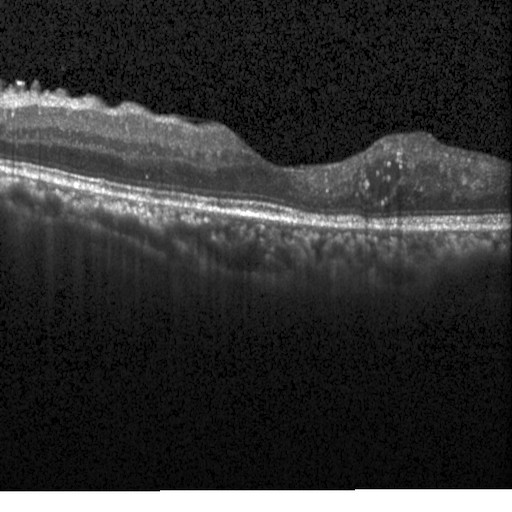 Retinal OCT cross-section · horizontal scan through the fovea · spectral-domain optical coherence tomography · Heidelberg Spectralis
DME.